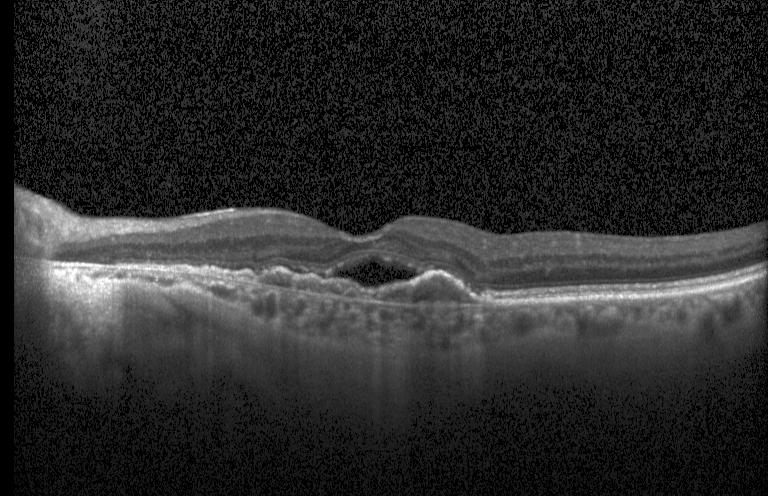
Spectral-domain OCT, optical coherence tomography scan — Finding: choroidal neovascularization (CNV).